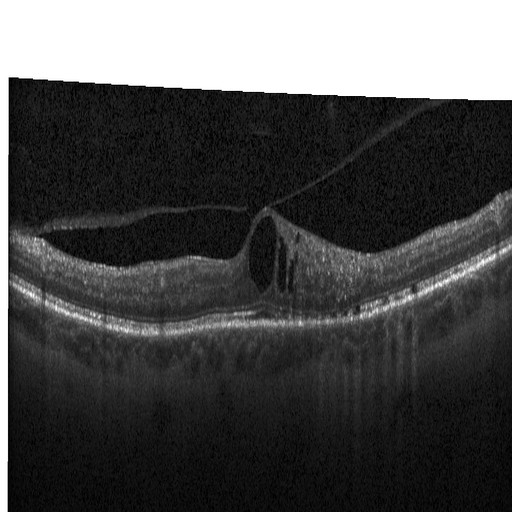 Finding: DME.